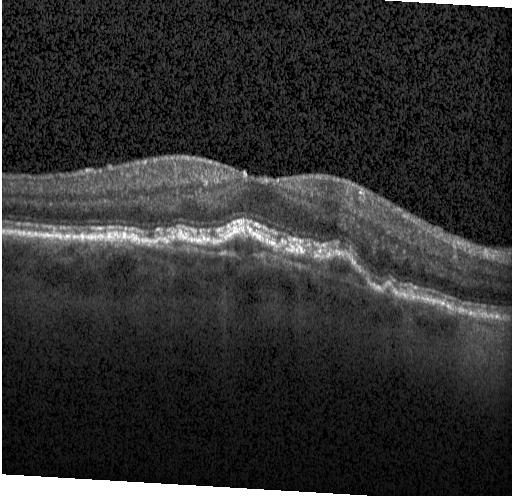
OCT line scan; instrument: Heidelberg Spectralis; SD-OCT
A choroidal neovascular membrane.